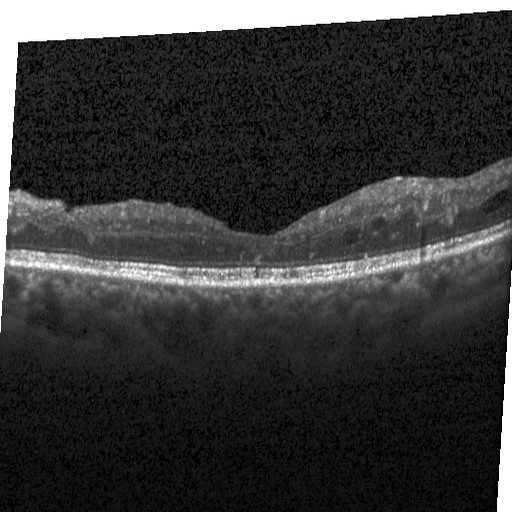 Spectral-domain optical coherence tomography, horizontal scan through the fovea, optical coherence tomography B-scan, Heidelberg Spectralis OCT system
Assessment: DME.